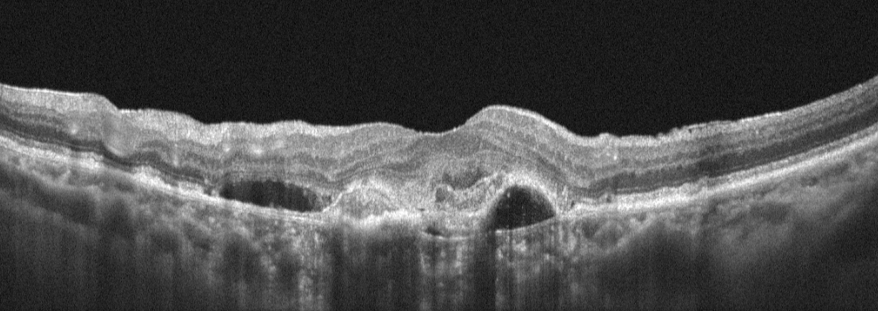

Macular OCT demonstrating AMD.